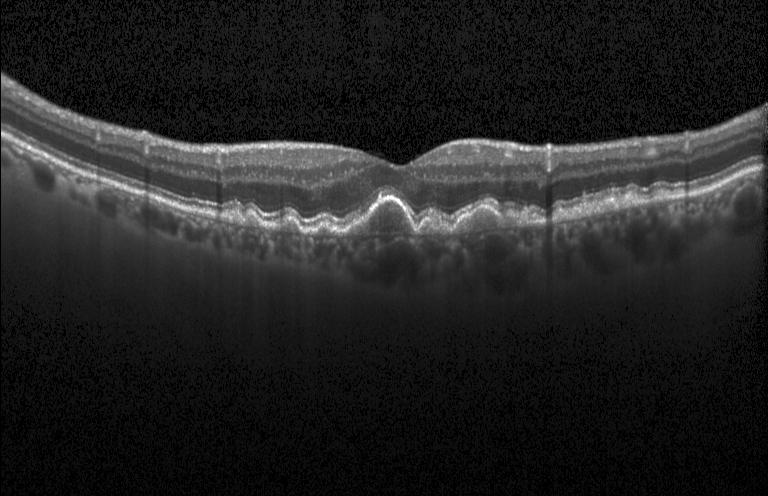
Retinal OCT B-scan. Spectral-domain OCT — OCT finding: drusen.